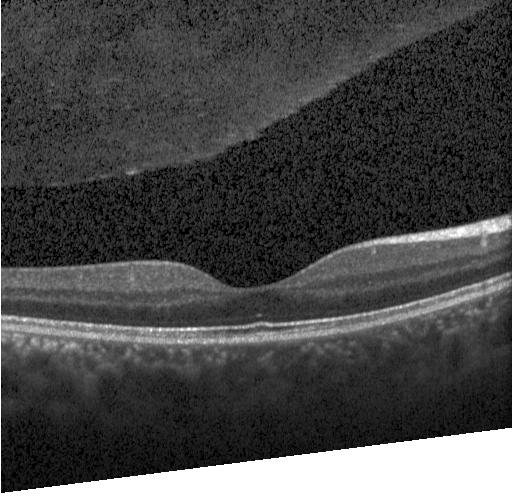
Heidelberg Spectralis, optical coherence tomography B-scan, spectral-domain OCT — No evidence of choroidal neovascularization, diabetic macular edema, or drusen.